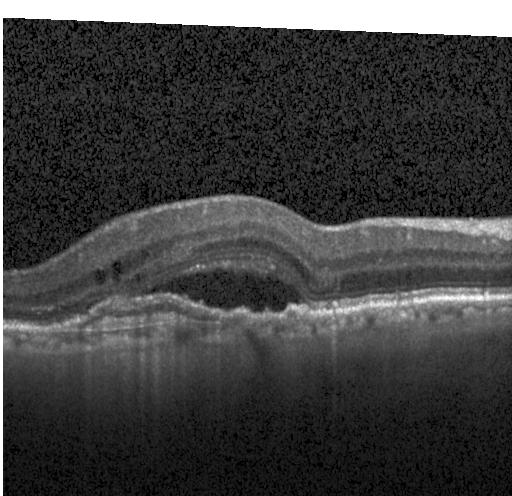

Impression: a choroidal neovascular membrane.